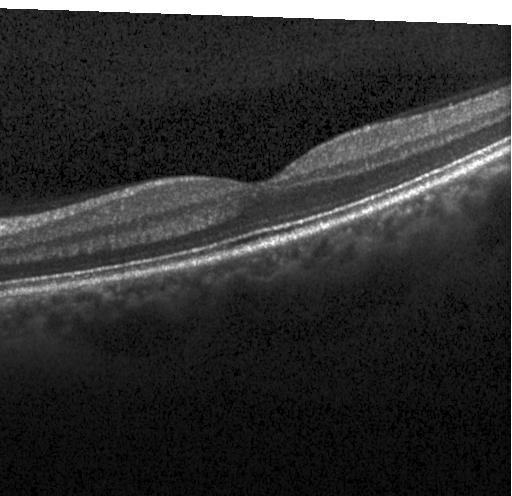 Instrument: Heidelberg Spectralis; optical coherence tomography B-scan; SD-OCT — Diagnosis: no evidence of choroidal neovascularization, diabetic macular edema, or drusen.